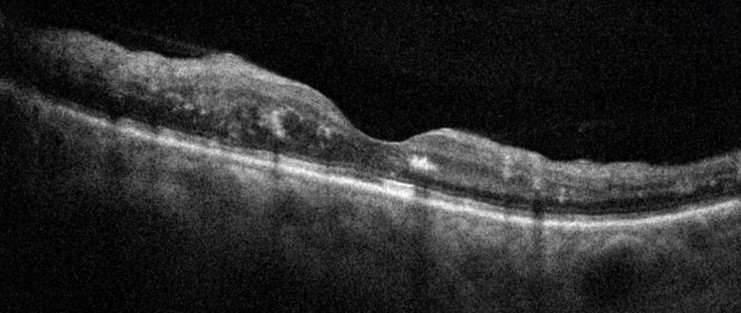

Instrument: Optovue Avanti RTVue XR; fovea-centered; retinal OCT B-scan.
Finding: DME.